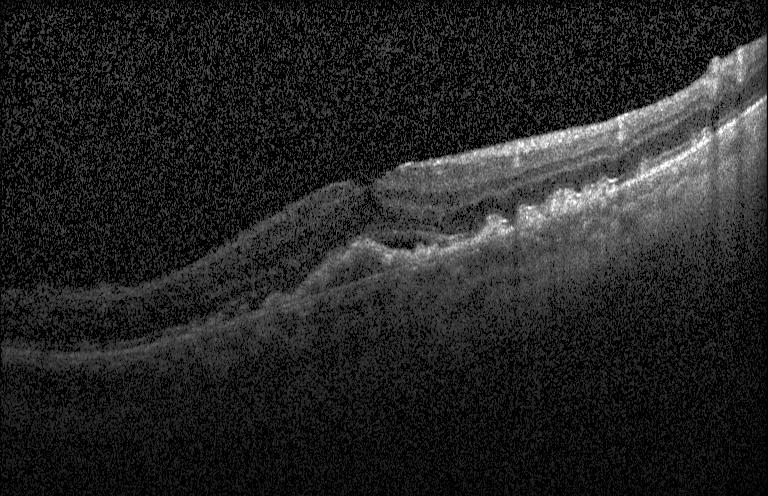

Optical coherence tomography scan
Impression: a choroidal neovascular membrane.